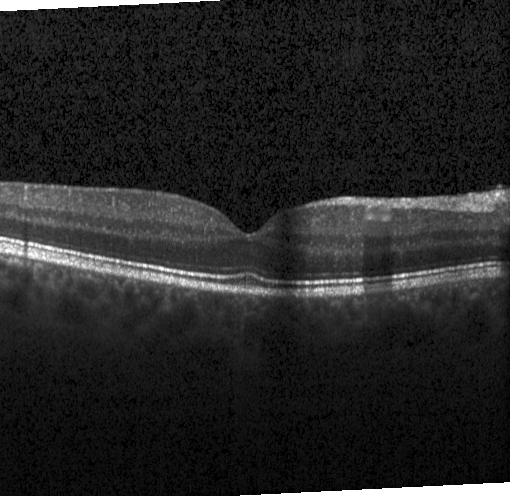 SD-OCT · Heidelberg Spectralis OCT system · optical coherence tomography B-scan · fovea-centered — Impression: no evidence of CNV, DME, or drusen.